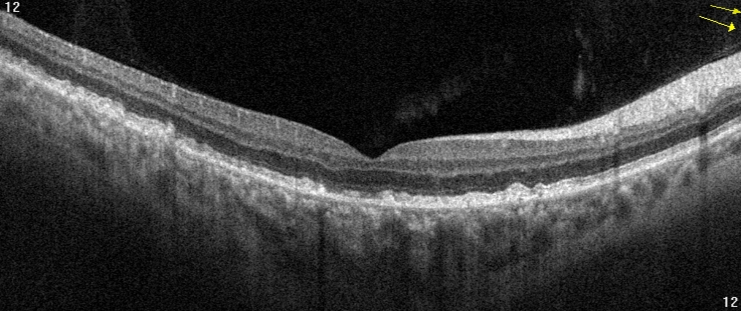 Retinal OCT B-scan. Impression: age-related macular degeneration (AMD).